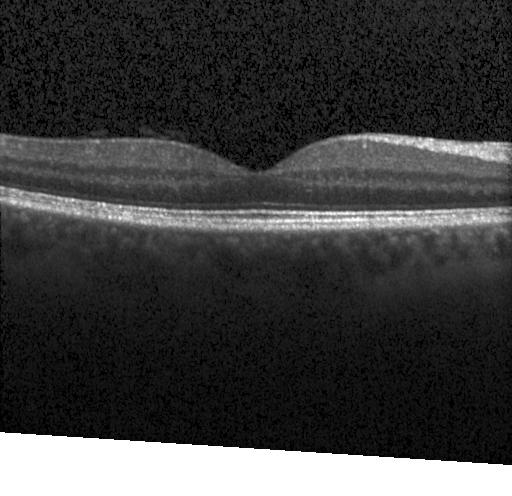 OCT B-scan · Heidelberg Spectralis · spectral-domain OCT — The scan shows no evidence of choroidal neovascularization, diabetic macular edema, or drusen.